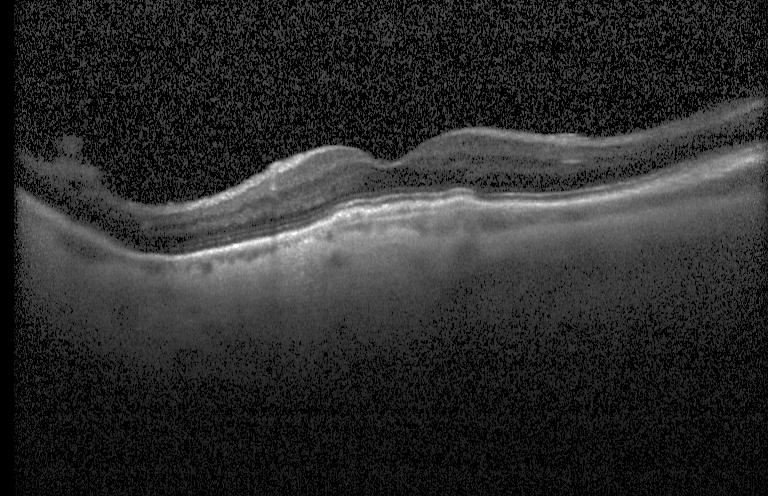 Spectral-domain optical coherence tomography. Instrument: Heidelberg Spectralis. OCT line scan — Assessment: CNV.